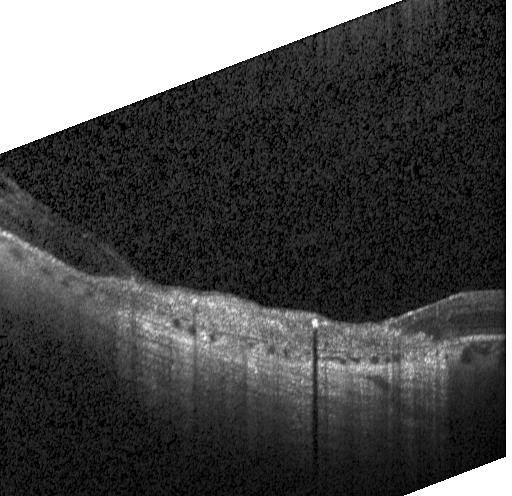
Assessment: CNV.